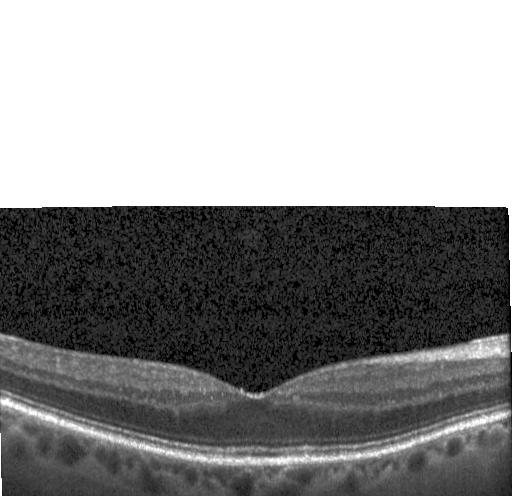 Dx: no evidence of CNV, DME, or drusen.